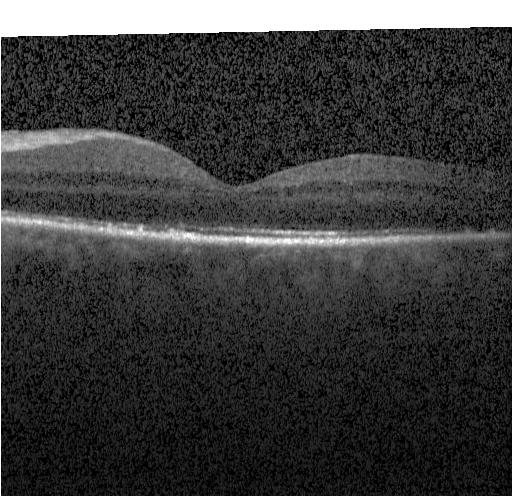

Dx: no evidence of choroidal neovascularization, diabetic macular edema, or drusen.